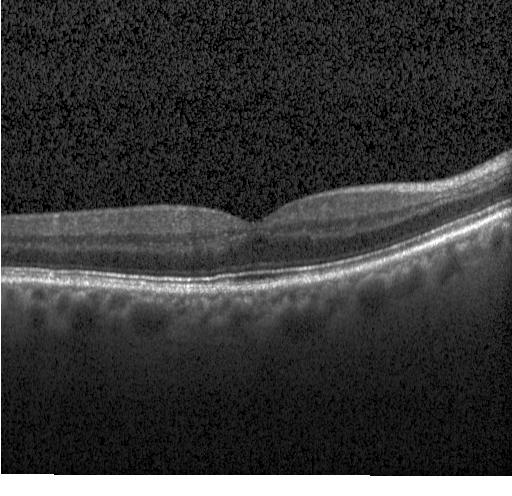 Spectral-domain OCT B-scan: no evidence of choroidal neovascularization, diabetic macular edema, or drusen.